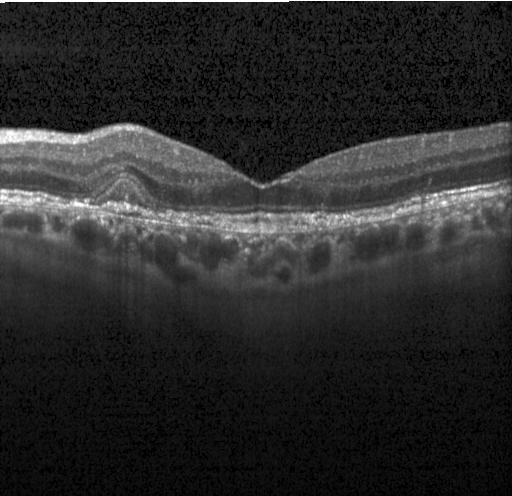

SD-OCT · optical coherence tomography scan · acquired on a Heidelberg Spectralis — Finding: multiple drusen.